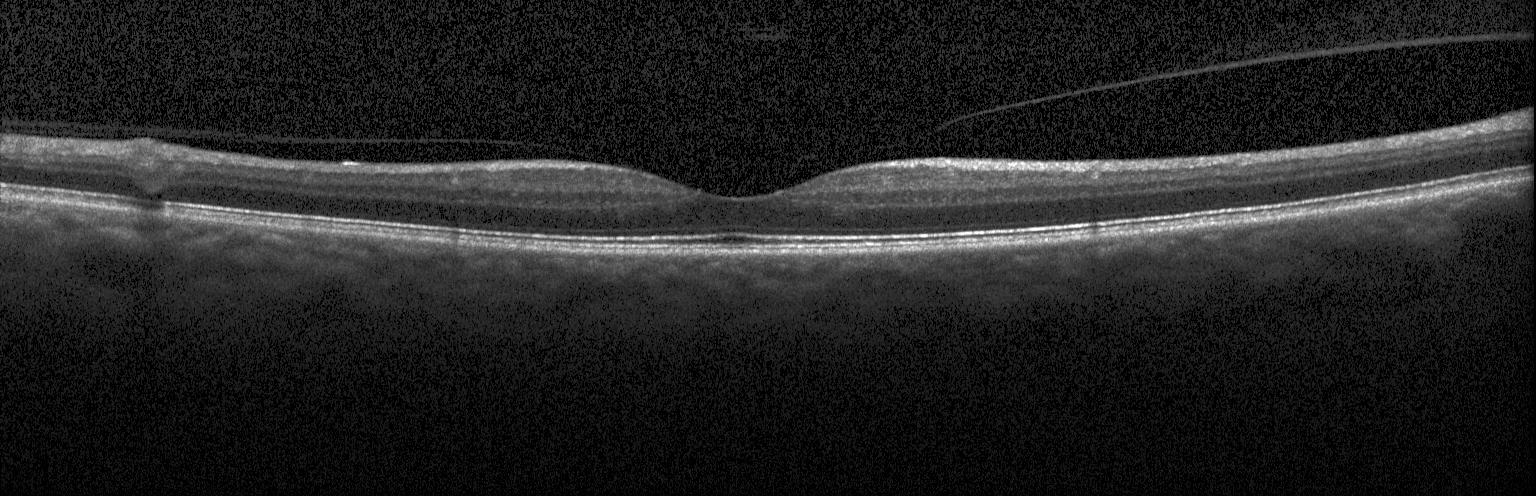

Centered on the fovea; spectral-domain optical coherence tomography; OCT B-scan; instrument: Heidelberg Spectralis
Impression: no choroidal neovascularization, diabetic macular edema, or drusen.